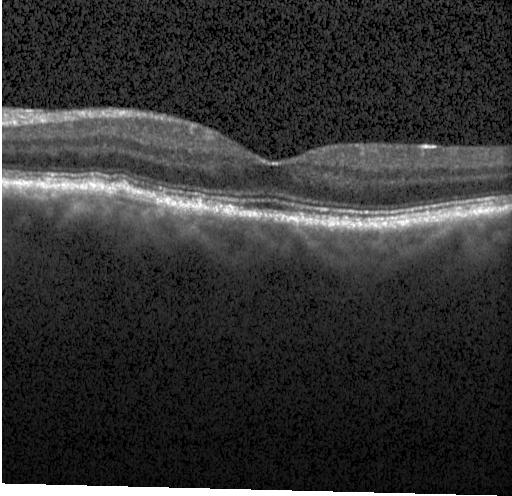 Assessment: multiple drusen.